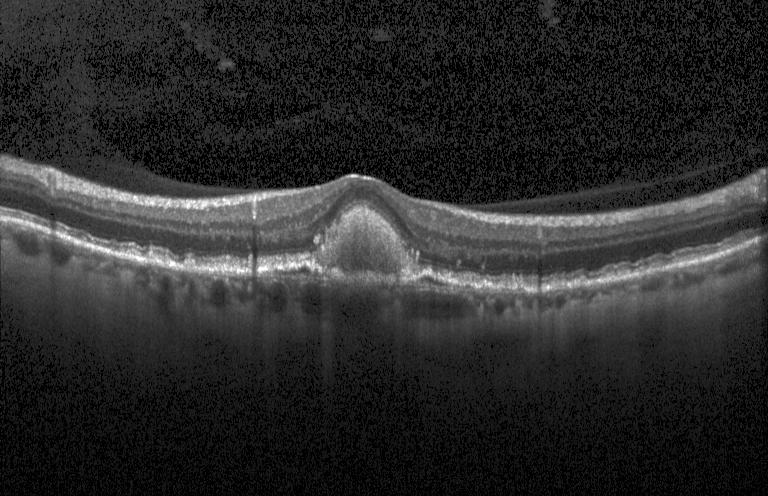 OCT finding: choroidal neovascularization.